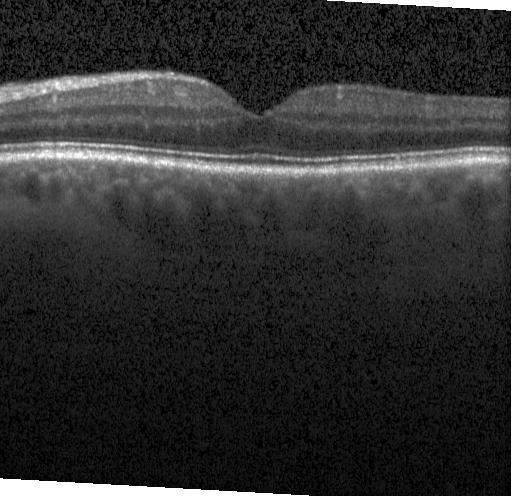

SD-OCT; Heidelberg Spectralis OCT system; retinal OCT B-scan
Finding: neither CNV, DME, nor drusen.